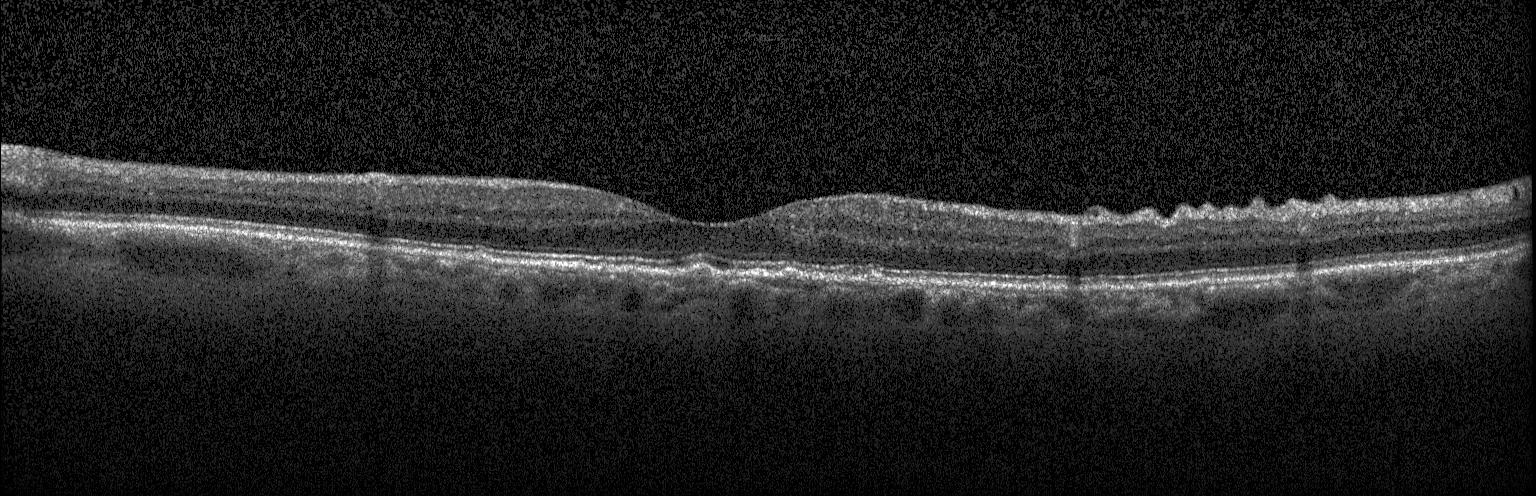 Impression: drusen.